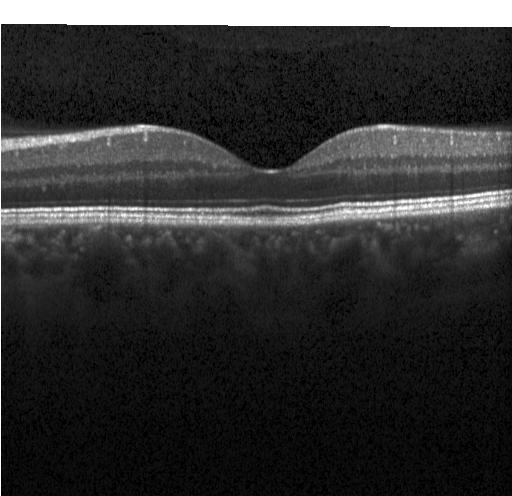
OCT scan showing neither choroidal neovascularization, diabetic macular edema, nor drusen.